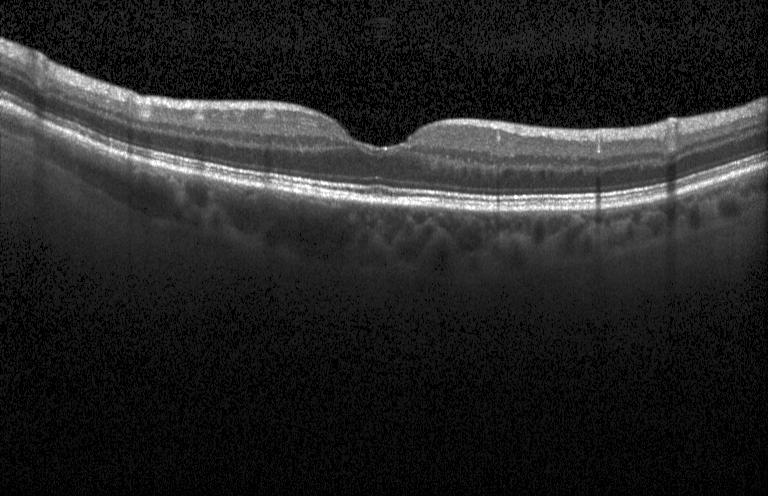
Heidelberg Spectralis OCT system, OCT line scan, spectral-domain optical coherence tomography
Dx: neither choroidal neovascularization, diabetic macular edema, nor drusen.